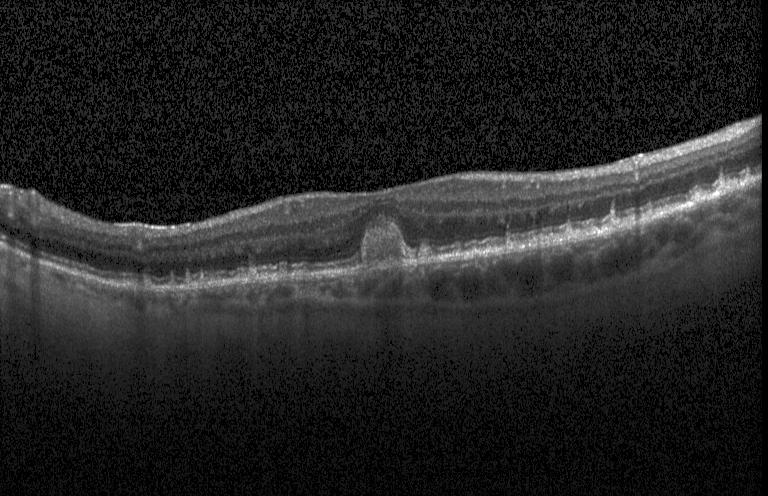
Impression: choroidal neovascularization.